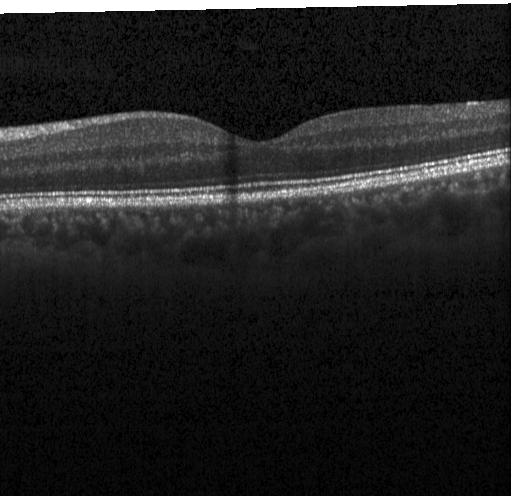
No choroidal neovascularization, diabetic macular edema, or drusen.